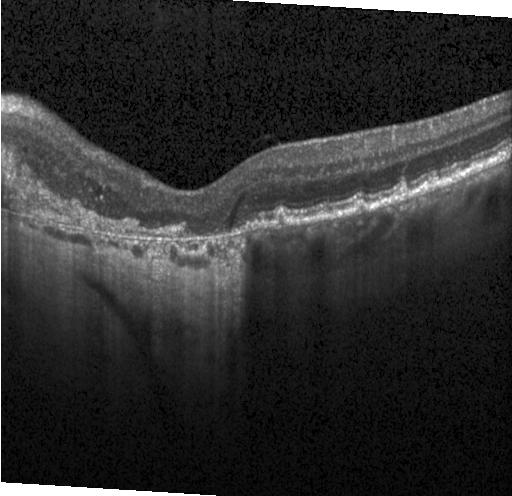 Finding: a choroidal neovascular membrane.